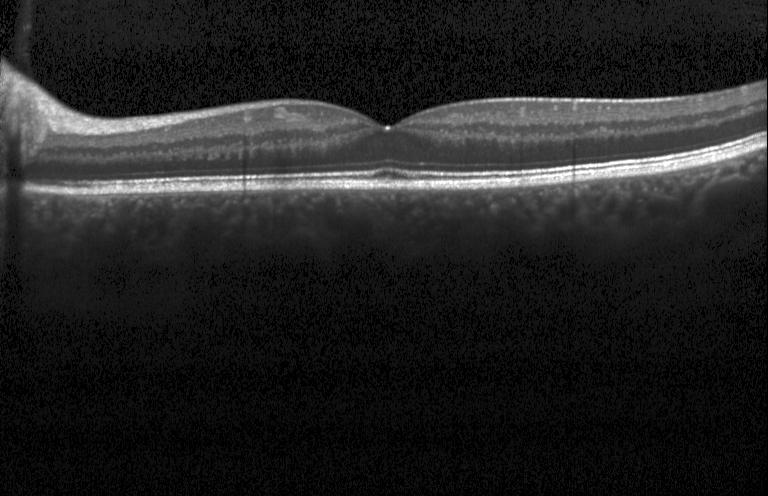 Macular OCT demonstrating no CNV, DME, or drusen.